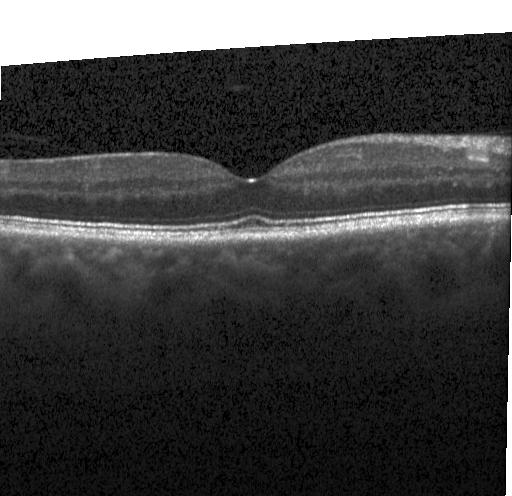
Impression: neither CNV, DME, nor drusen.